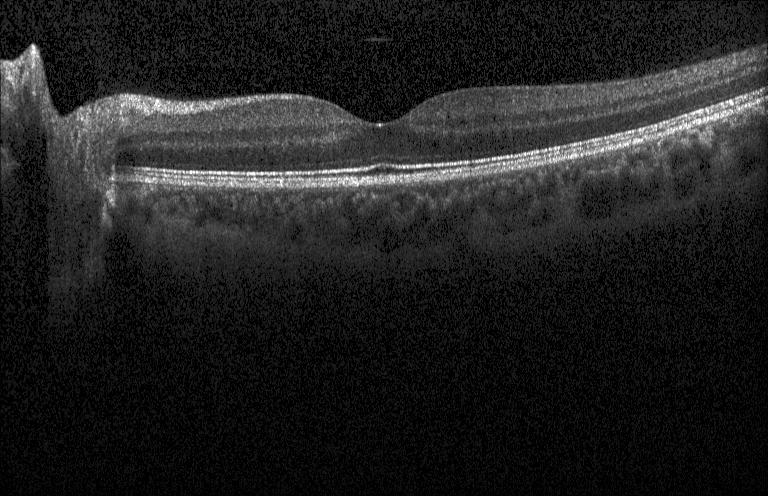

Retinal OCT B-scan · spectral-domain OCT · fovea-centered · Heidelberg Spectralis
Diagnosis: neither CNV, DME, nor drusen.